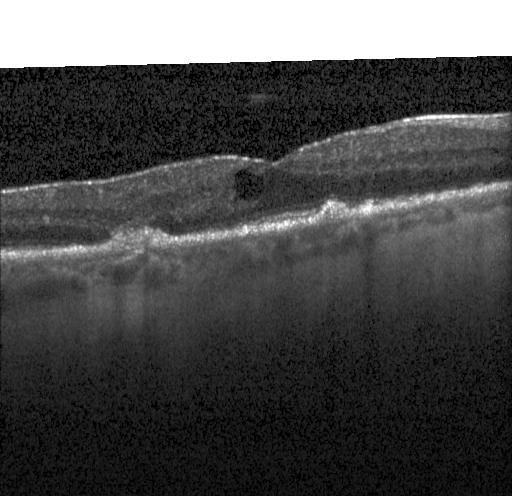 OCT finding: choroidal neovascularization.